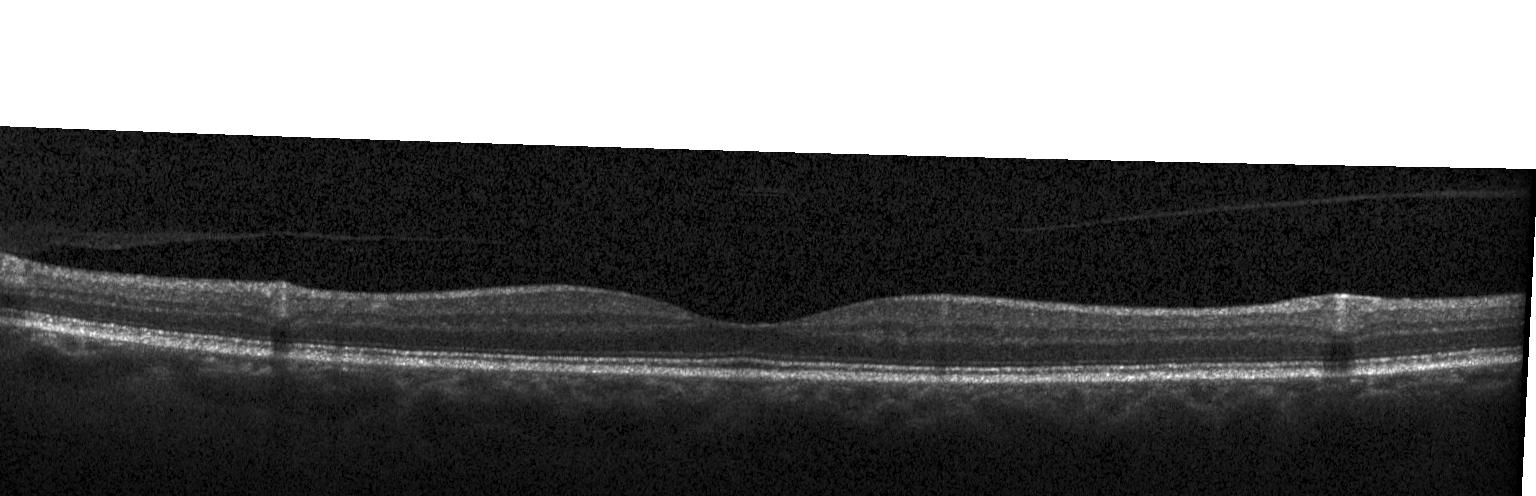

Optical coherence tomography scan, spectral-domain OCT, Heidelberg Spectralis, horizontal scan through the fovea
Assessment: no CNV, no DME, and no drusen.